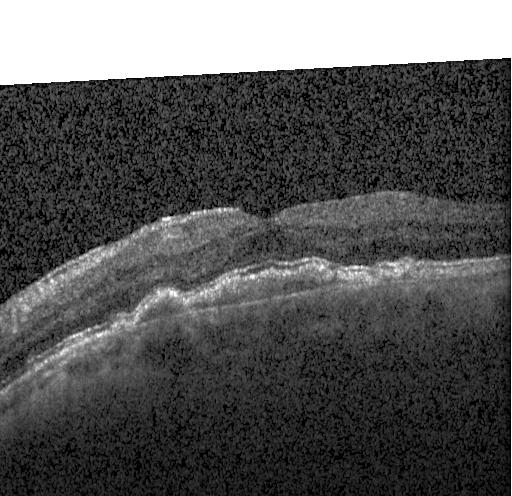
OCT finding: a choroidal neovascular membrane.